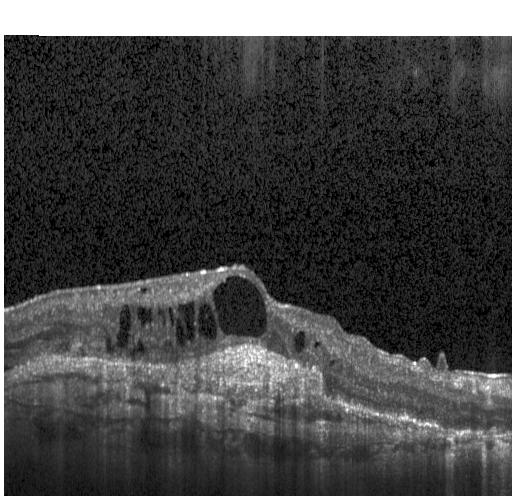

Diagnosis: CNV.